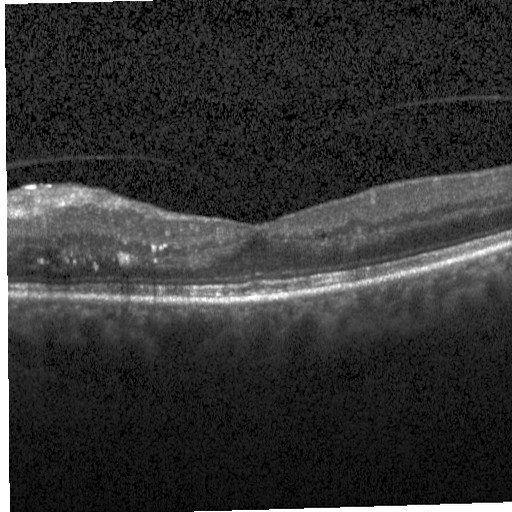

Spectral-domain optical coherence tomography; retinal OCT B-scan; macular scan; acquired on a Heidelberg Spectralis — Diabetic macular edema (DME).